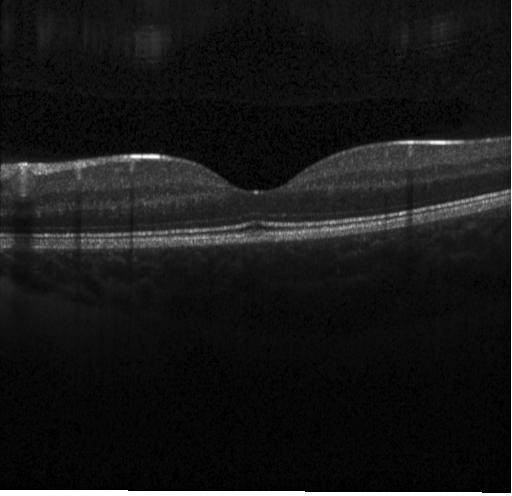

Retinal OCT B-scan
Dx: no CNV, no DME, and no drusen.